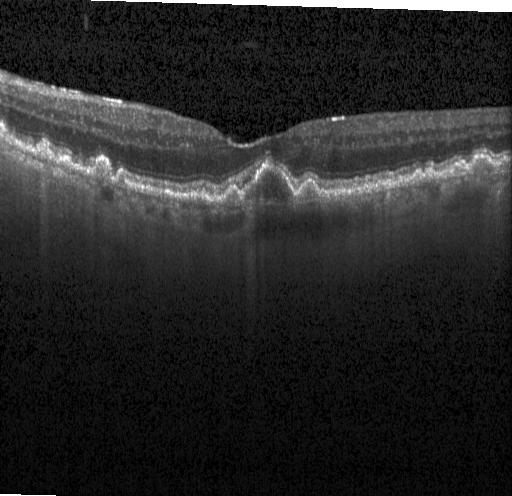 OCT line scan — Assessment: drusen.